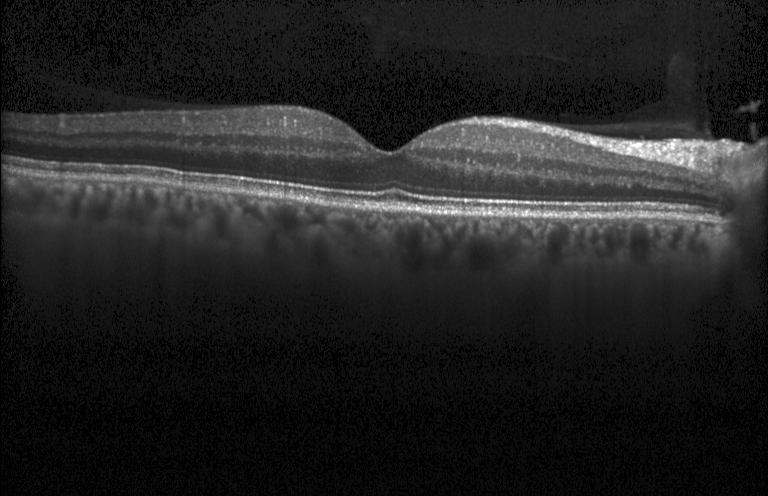
Spectral-domain OCT, optical coherence tomography scan, acquired on a Heidelberg Spectralis
Diagnosis: neither choroidal neovascularization, diabetic macular edema, nor drusen.